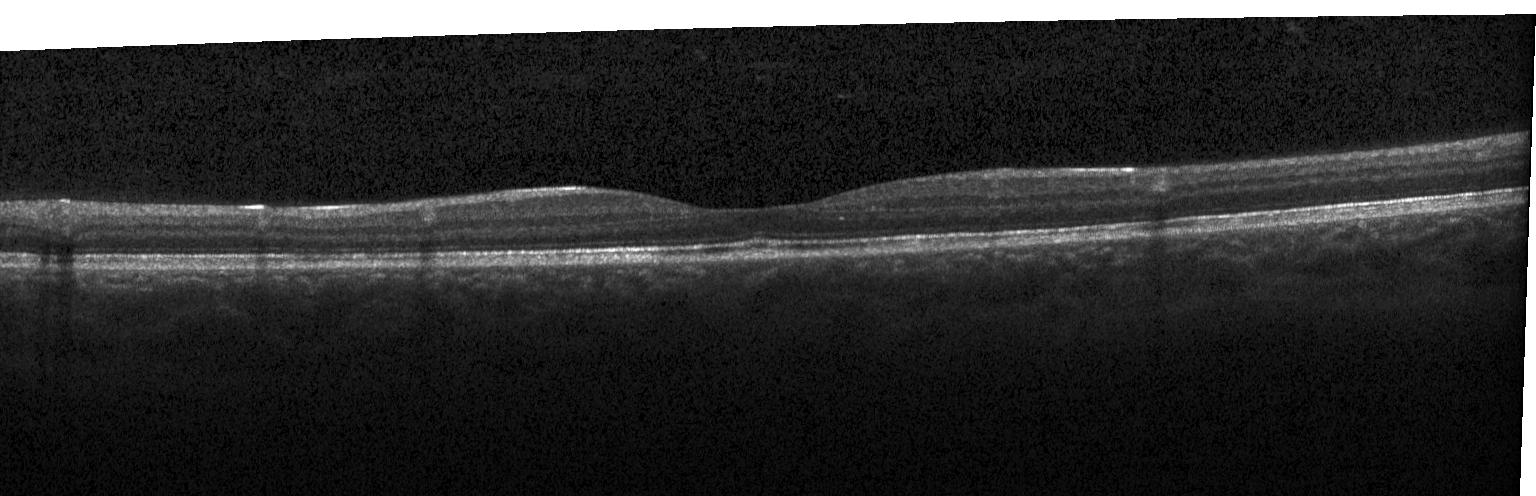 The scan shows no evidence of choroidal neovascularization, diabetic macular edema, or drusen.